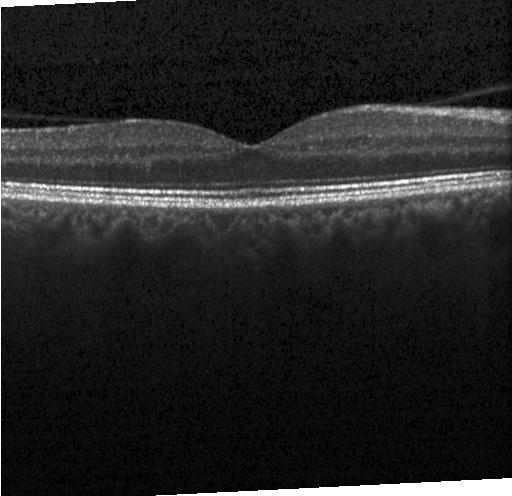 Retinal OCT cross-section.
Diagnosis: no choroidal neovascularization, no diabetic macular edema, and no drusen.